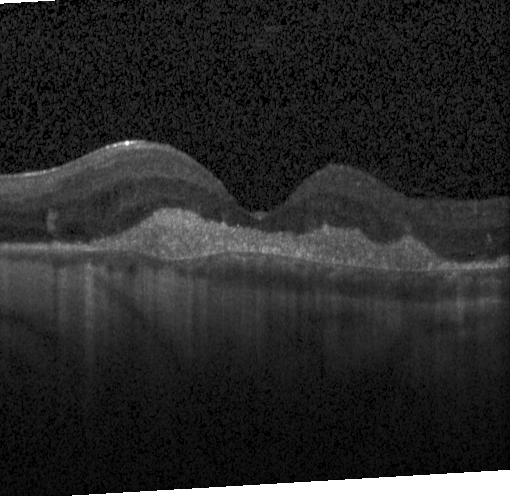
OCT finding: CNV.